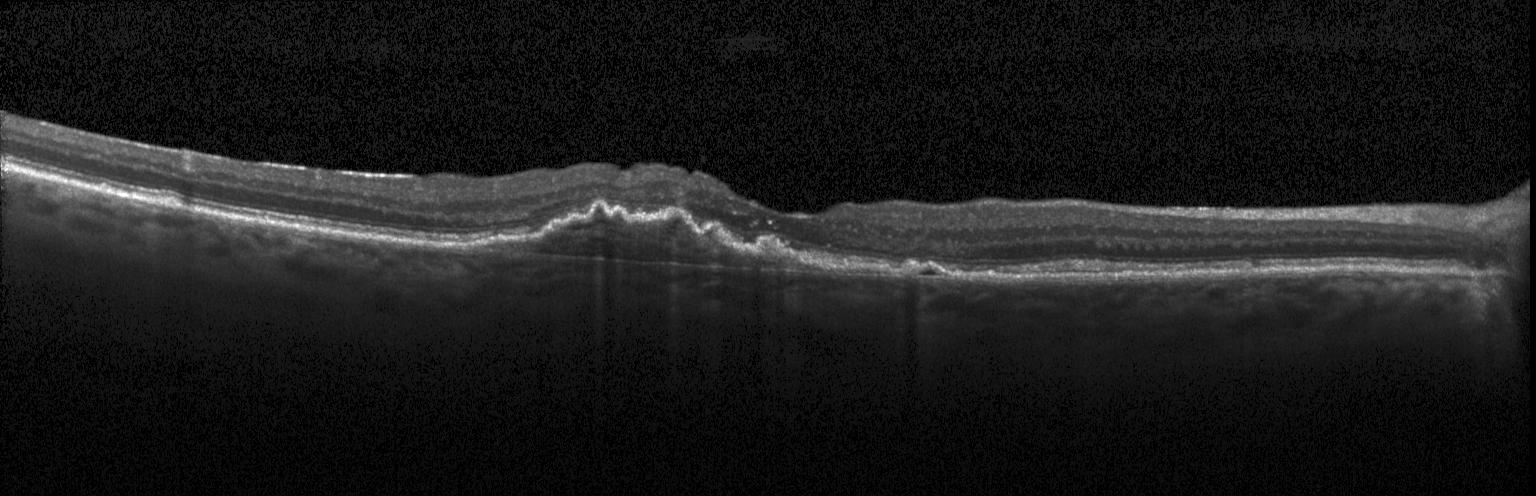

Retinal OCT cross-section showing a choroidal neovascular membrane.